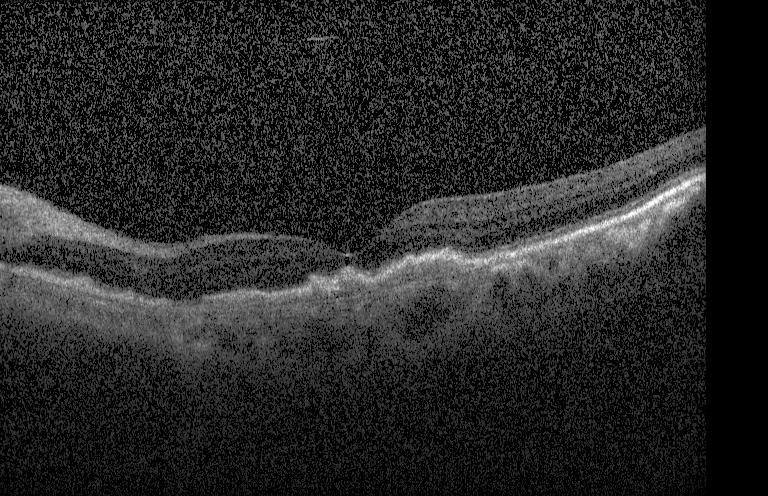
Choroidal neovascularization.